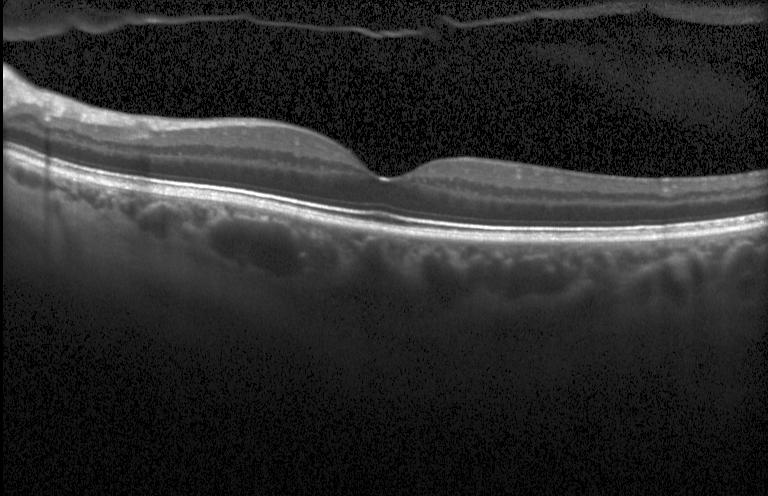 Macular OCT demonstrating no CNV, DME, or drusen.